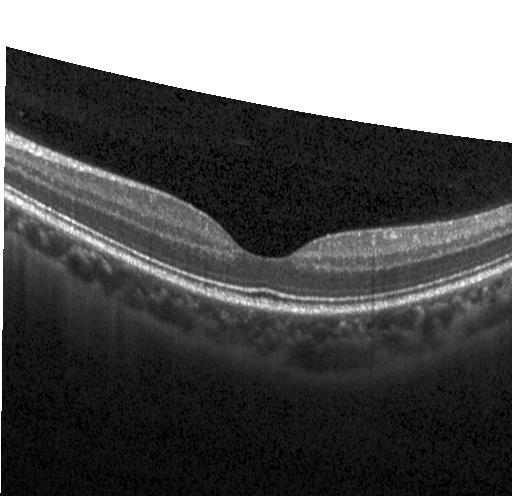 Impression: no choroidal neovascularization, diabetic macular edema, or drusen.